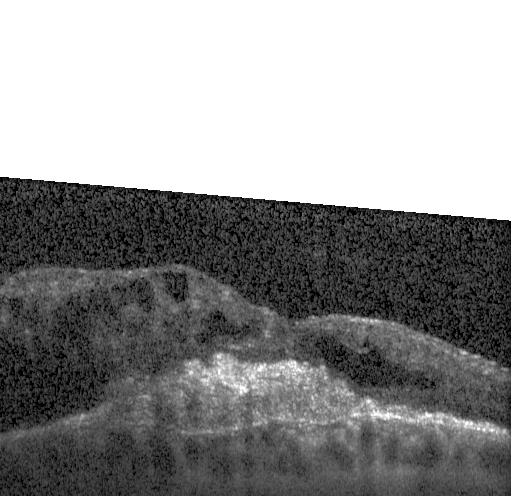

Assessment: a choroidal neovascular membrane.